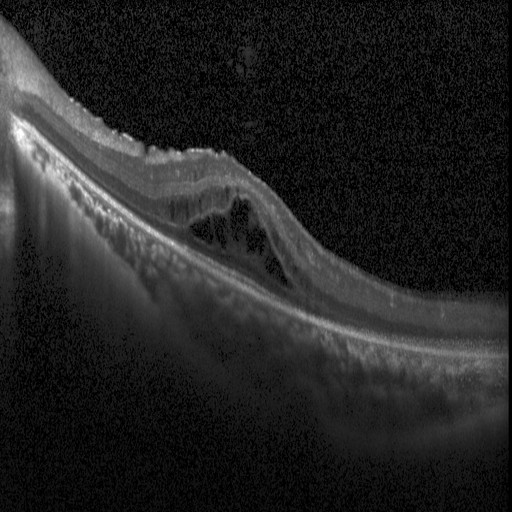
Assessment: DME.